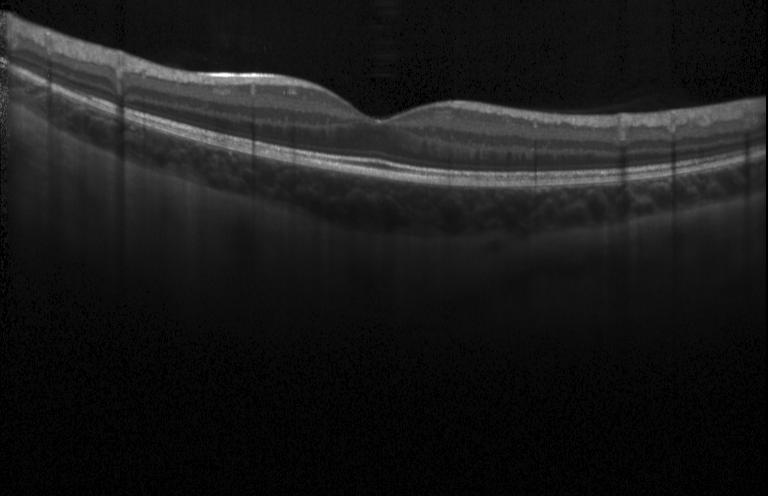 Retinal OCT cross-section
Impression: no CNV, DME, or drusen.